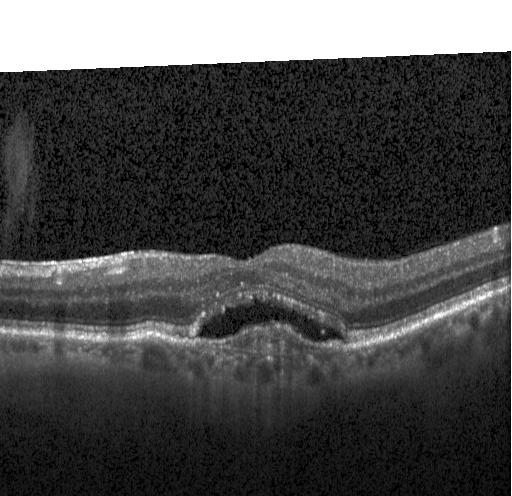 Retinal OCT cross-section. This B-scan demonstrates a choroidal neovascular membrane.